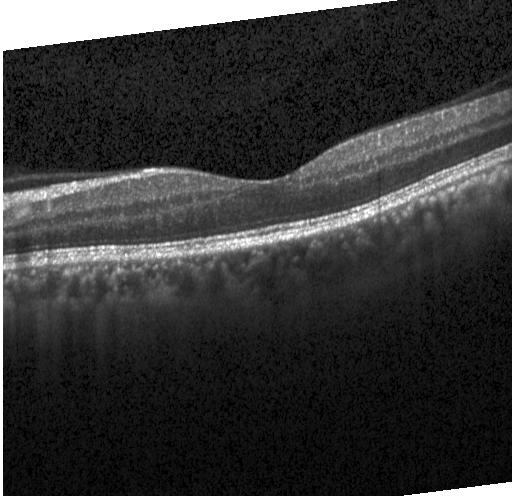 No choroidal neovascularization, no diabetic macular edema, and no drusen.